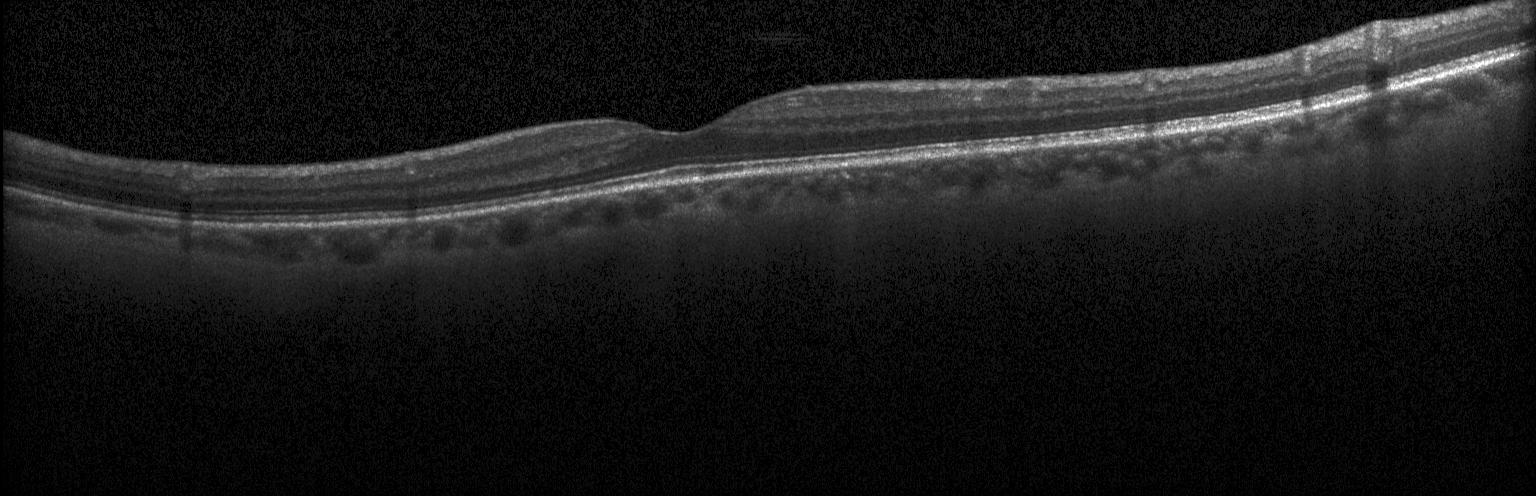 Optical coherence tomography B-scan, spectral-domain OCT, instrument: Heidelberg Spectralis
OCT finding: neither choroidal neovascularization, diabetic macular edema, nor drusen.